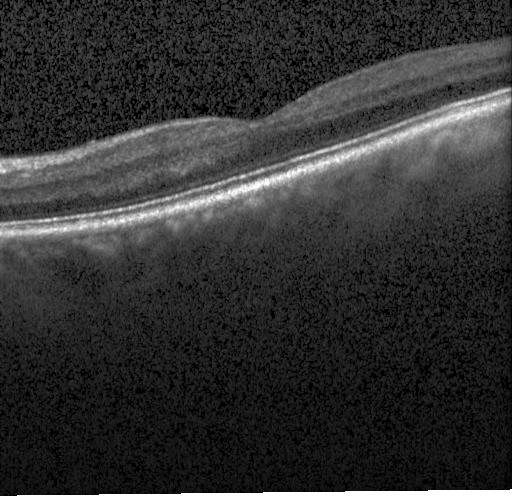 Impression: no choroidal neovascularization, diabetic macular edema, or drusen.